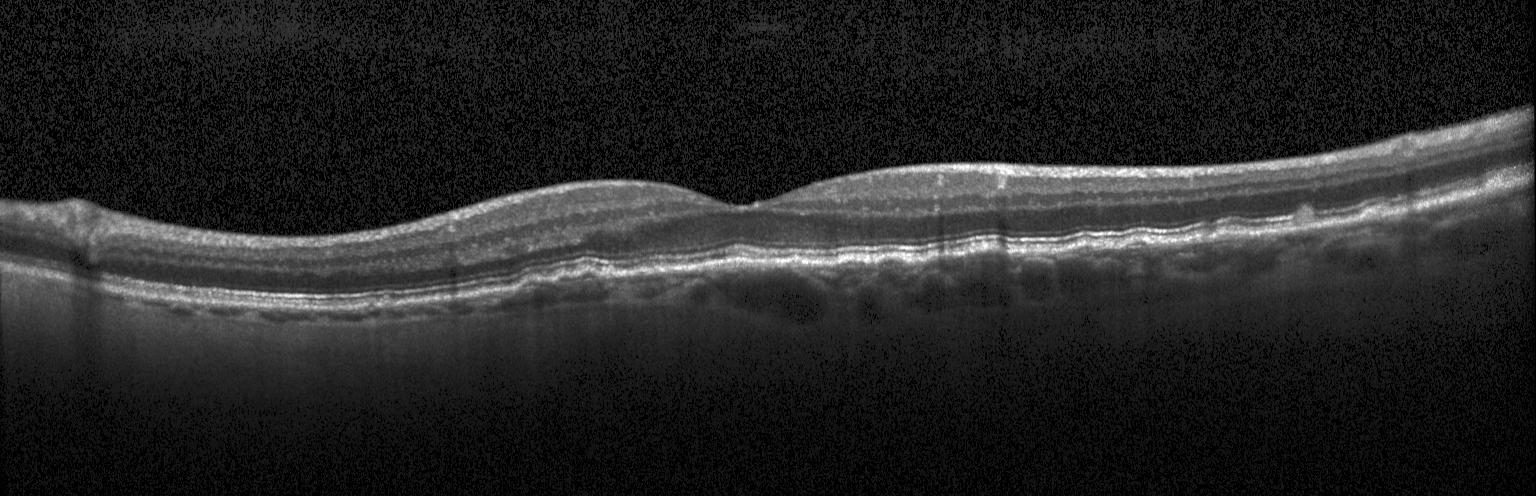
Fovea-centered. SD-OCT. Heidelberg Spectralis OCT system. Optical coherence tomography B-scan. Finding: sub-RPE drusenoid deposits.